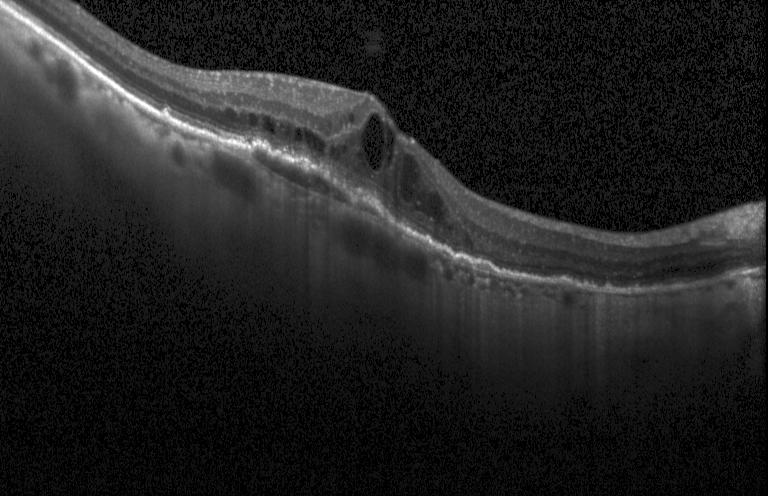
Retinal OCT B-scan, horizontal scan through the fovea, spectral-domain OCT. Diagnosis: a choroidal neovascular membrane.